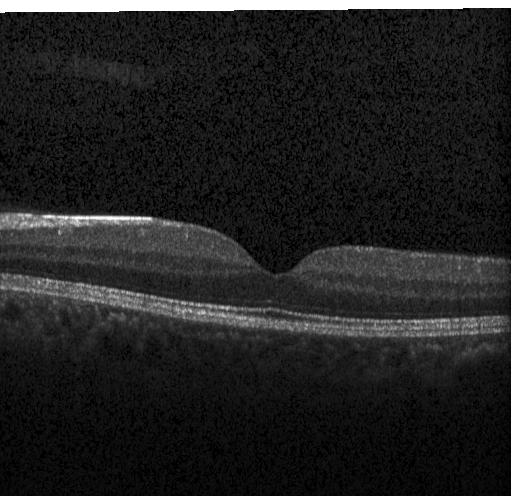

Retinal OCT cross-section.
Macular OCT: no evidence of CNV, DME, or drusen.